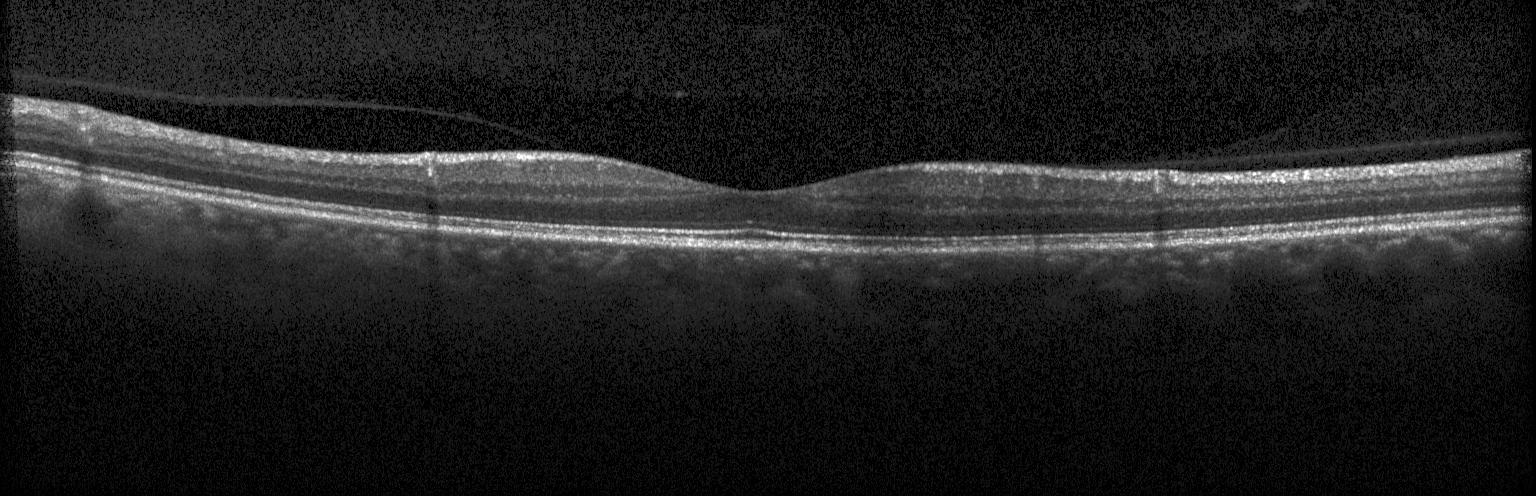

SD-OCT · OCT B-scan · Heidelberg Spectralis OCT system
Macular OCT: no CNV, no DME, and no drusen.